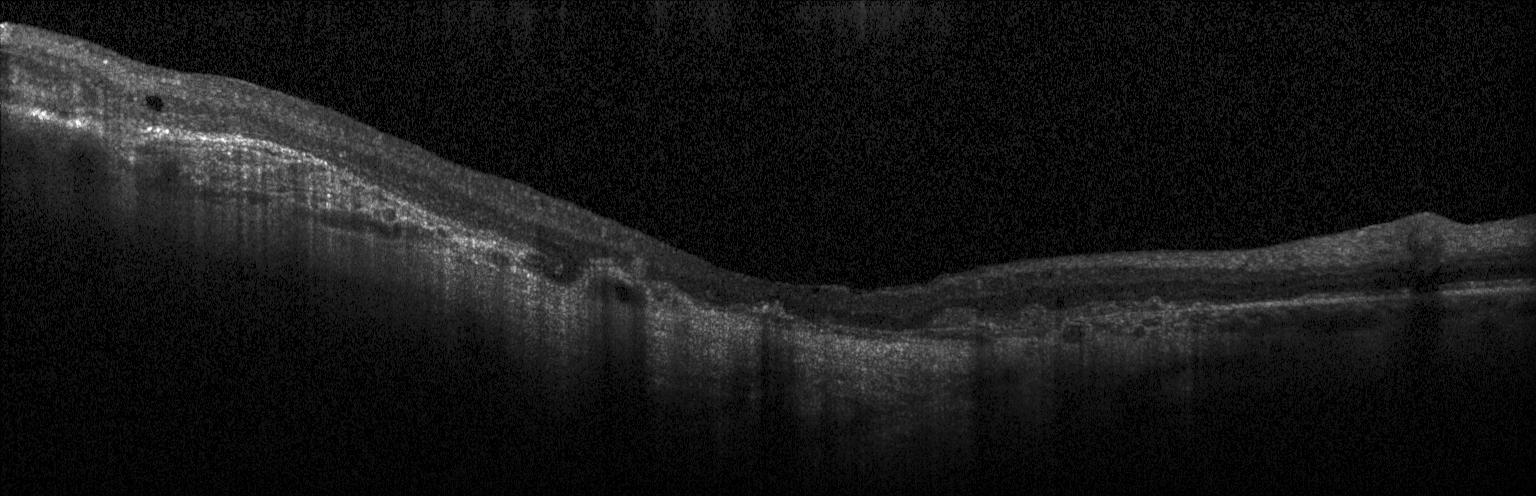

Optical coherence tomography scan — The scan shows CNV.